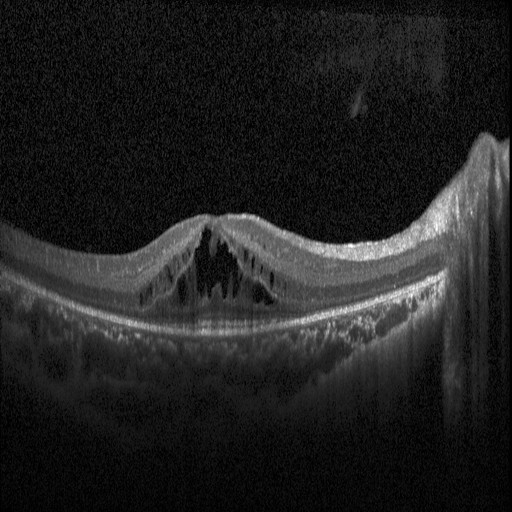
Retinal OCT B-scan · centered on the fovea · spectral-domain OCT — Assessment: DME.